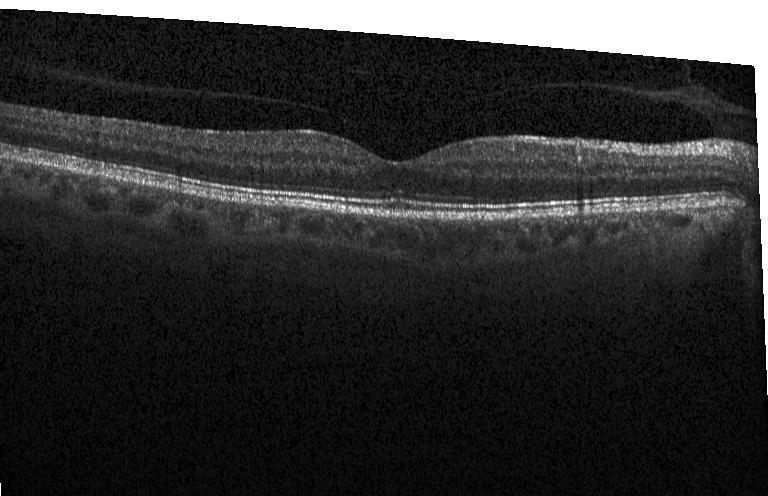

Retinal OCT B-scan
The scan shows no evidence of choroidal neovascularization, diabetic macular edema, or drusen.